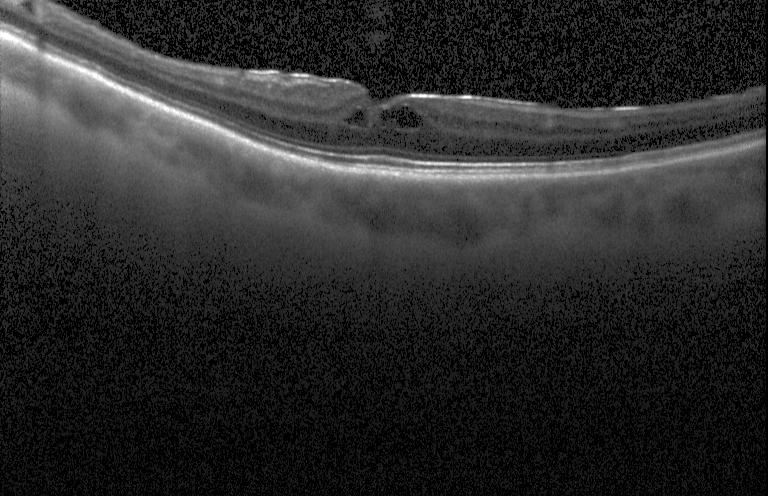 Macular OCT demonstrating DME.